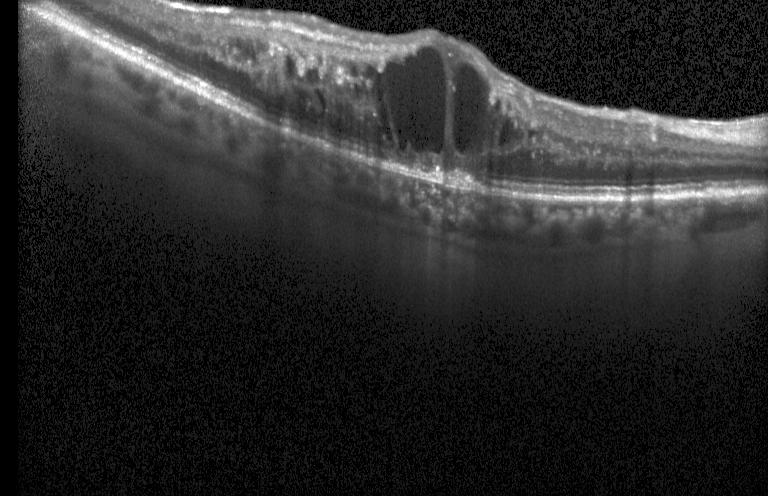

Optical coherence tomography B-scan, Heidelberg Spectralis OCT system.
The scan shows a choroidal neovascular membrane.